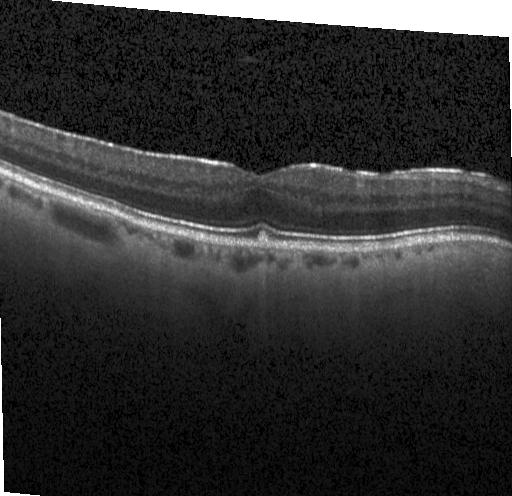
Heidelberg Spectralis · retinal OCT cross-section · centered on the fovea — Diagnosis: drusen.